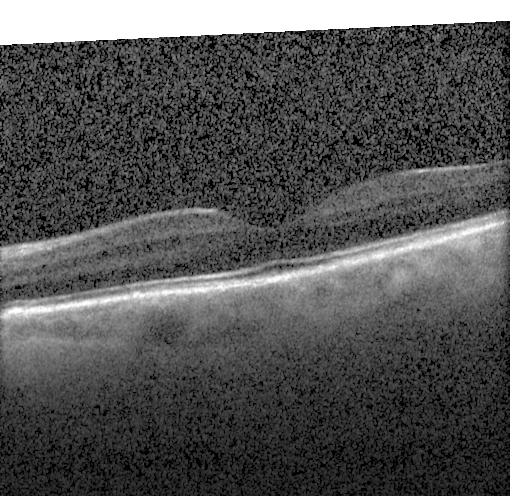
No CNV, DME, or drusen.